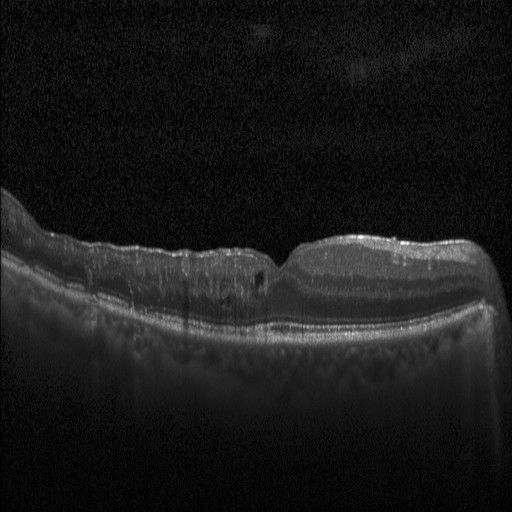
Retinal OCT B-scan; Heidelberg Spectralis; macular scan. Diagnosis: diabetic macular edema.